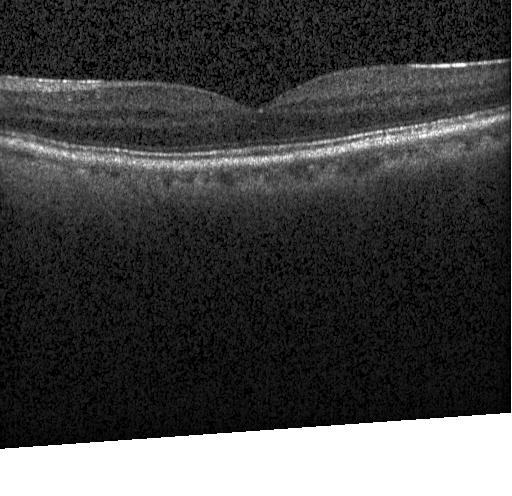
Instrument: Heidelberg Spectralis, retinal OCT B-scan
Assessment: no evidence of CNV, DME, or drusen.